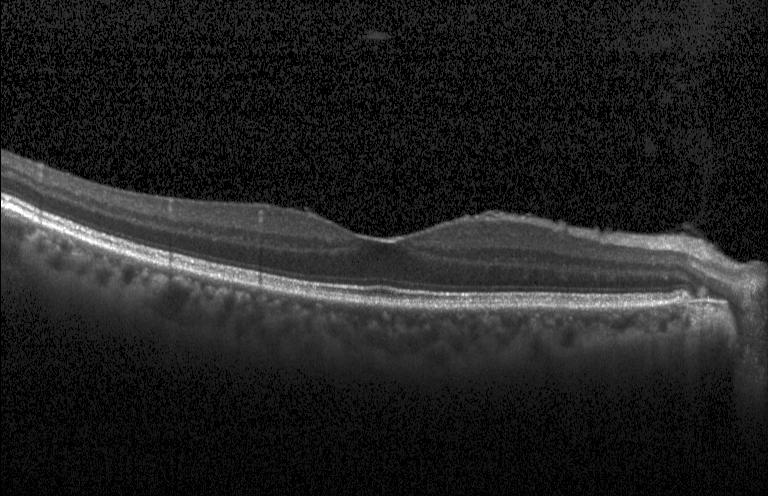
Spectral-domain optical coherence tomography. Retinal OCT B-scan. Heidelberg Spectralis OCT system — The scan shows neither CNV, DME, nor drusen.